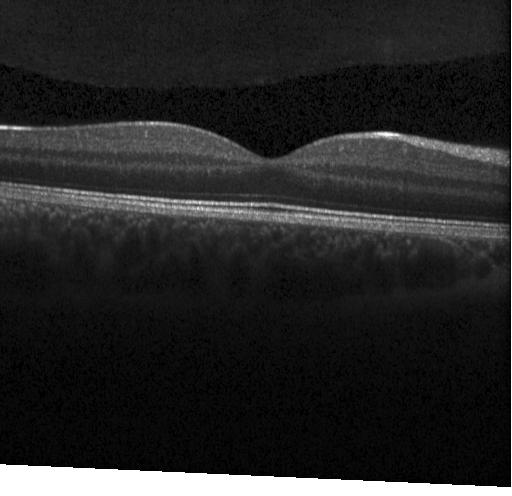 Through the macula · OCT line scan · Heidelberg Spectralis. Diagnosis: neither choroidal neovascularization, diabetic macular edema, nor drusen.